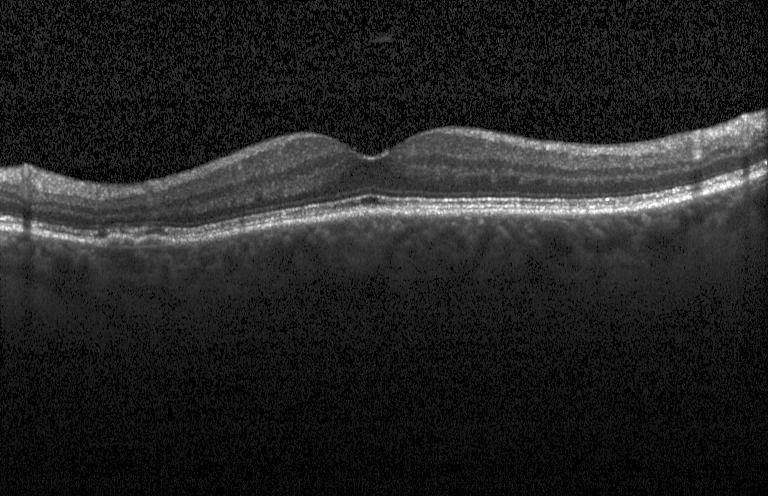
Macular scan · OCT B-scan · spectral-domain optical coherence tomography — This B-scan demonstrates a choroidal neovascular membrane.